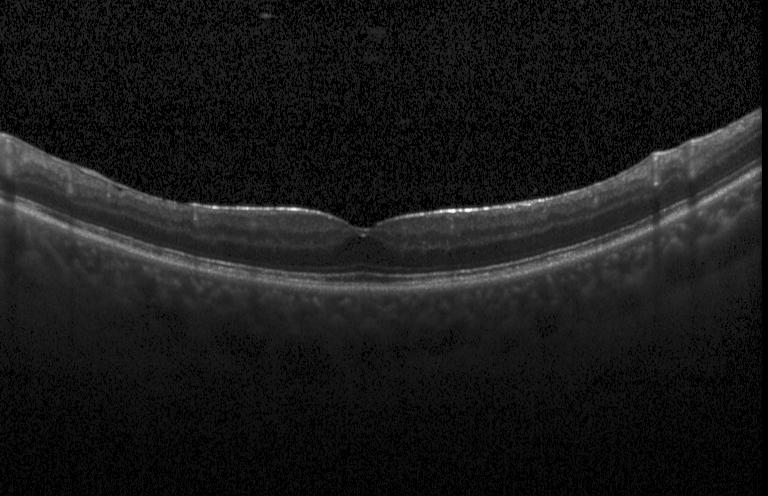 Centered on the fovea; retinal OCT B-scan; SD-OCT; Heidelberg Spectralis OCT system.
Dx: no evidence of choroidal neovascularization, diabetic macular edema, or drusen.